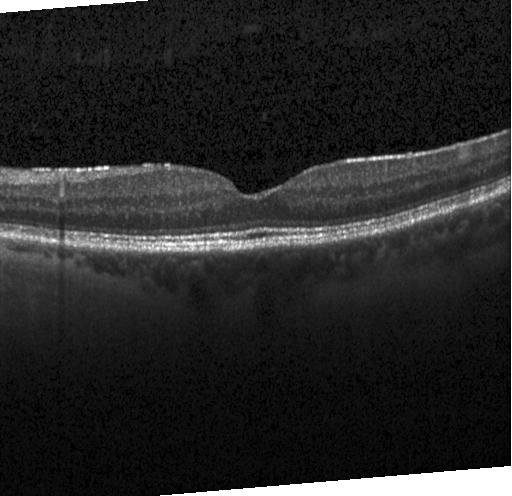 Macular OCT: no evidence of CNV, DME, or drusen.